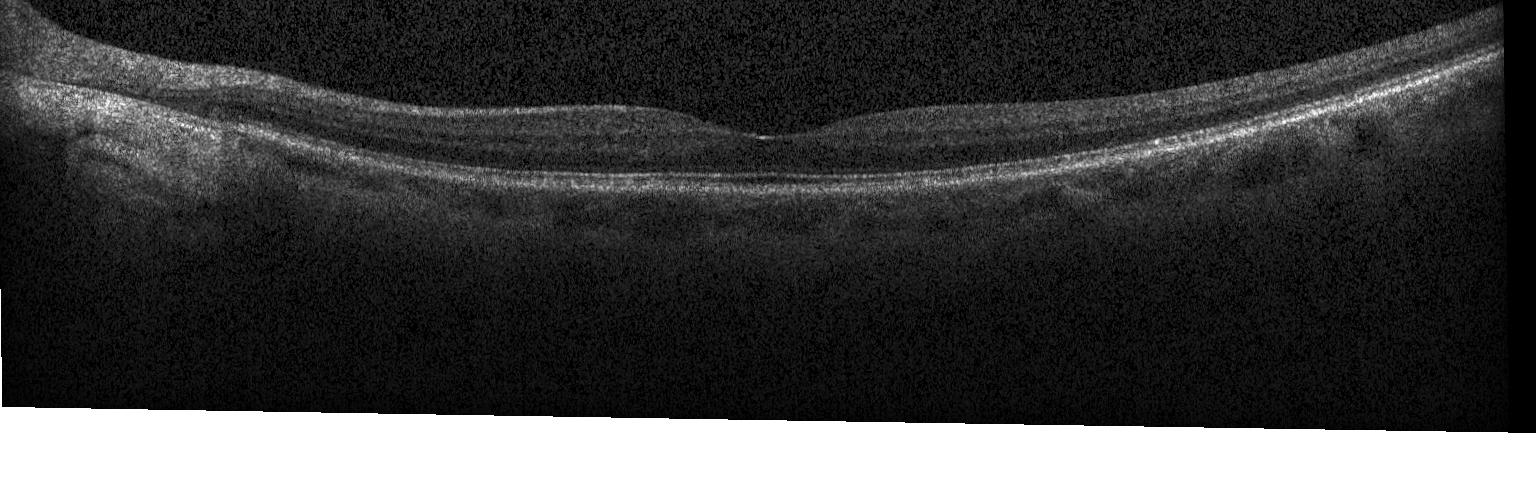

Instrument: Heidelberg Spectralis; optical coherence tomography B-scan — Finding: no choroidal neovascularization, diabetic macular edema, or drusen.